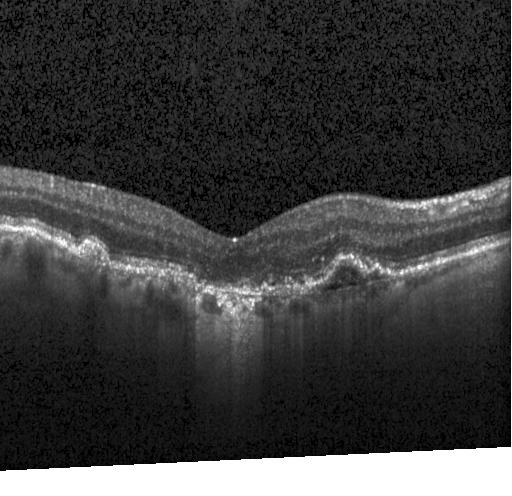
Macular OCT: a choroidal neovascular membrane.